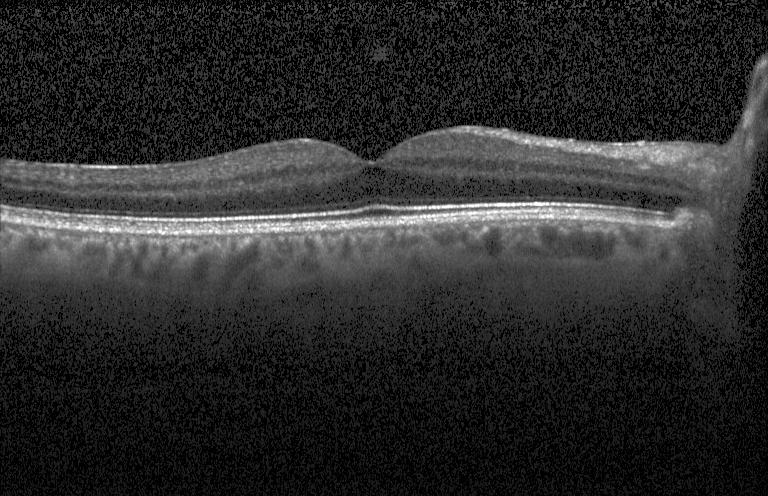
SD-OCT · horizontal scan through the fovea · retinal OCT B-scan. Diagnosis: neither choroidal neovascularization, diabetic macular edema, nor drusen.